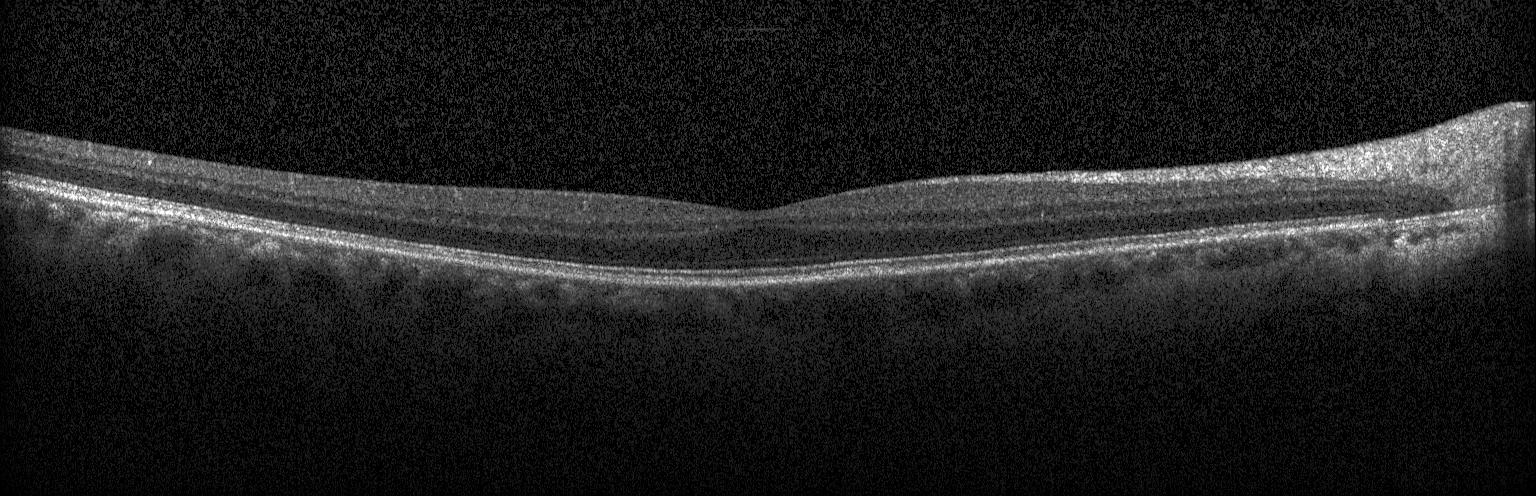
Spectral-domain OCT; fovea-centered; acquired on a Heidelberg Spectralis; retinal OCT cross-section
Diagnosis: neither CNV, DME, nor drusen.